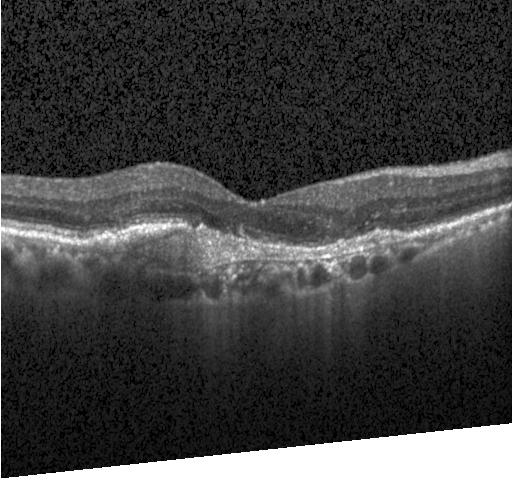
This B-scan demonstrates a choroidal neovascular membrane.